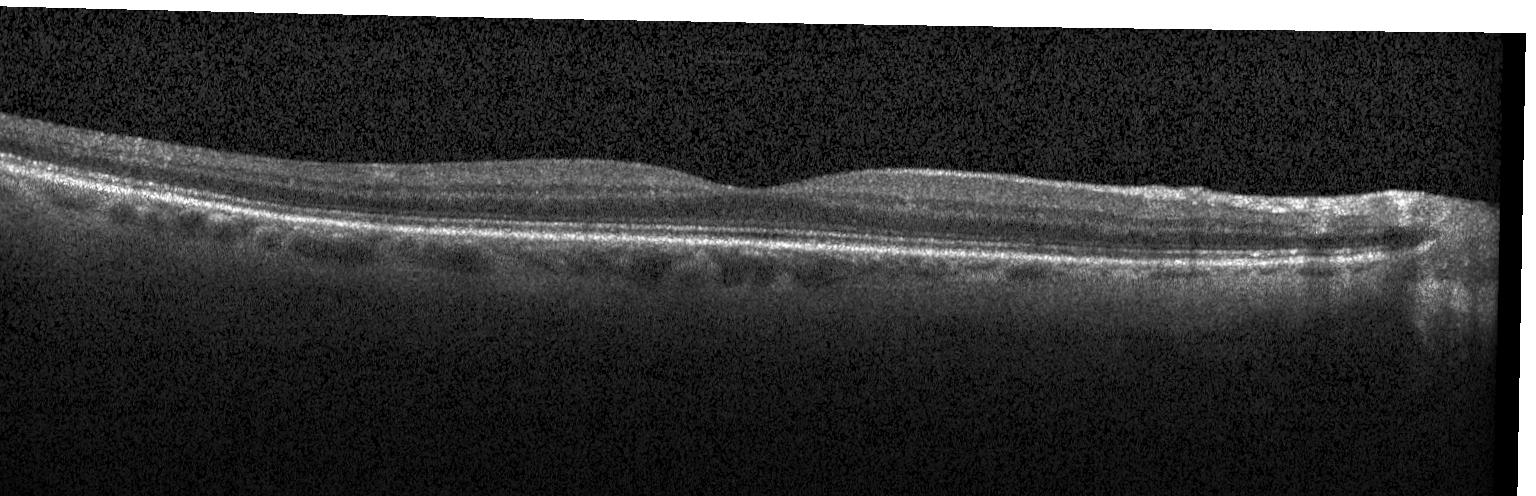

OCT B-scan; spectral-domain OCT; instrument: Heidelberg Spectralis — Impression: no evidence of choroidal neovascularization, diabetic macular edema, or drusen.